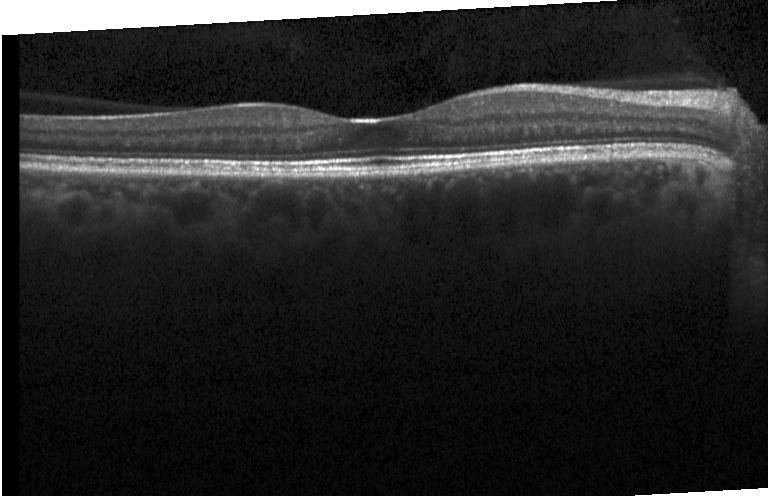
Heidelberg Spectralis OCT system; horizontal scan through the fovea; SD-OCT; retinal OCT B-scan.
Finding: no choroidal neovascularization, diabetic macular edema, or drusen.